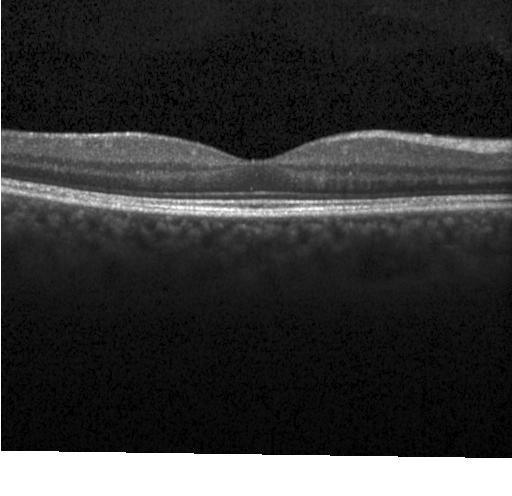

OCT line scan.
The scan shows no choroidal neovascularization, diabetic macular edema, or drusen.